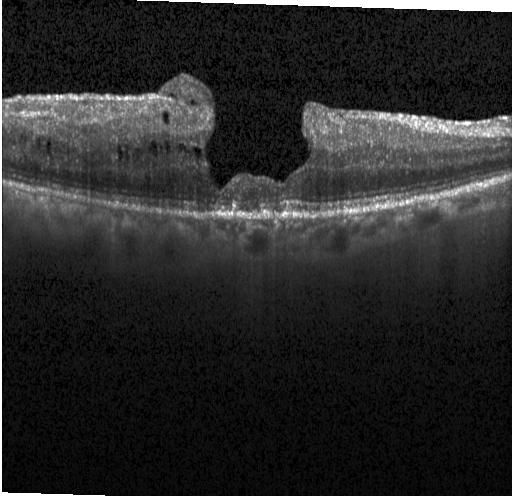
OCT B-scan, horizontal scan through the fovea.
Impression: diabetic macular edema.